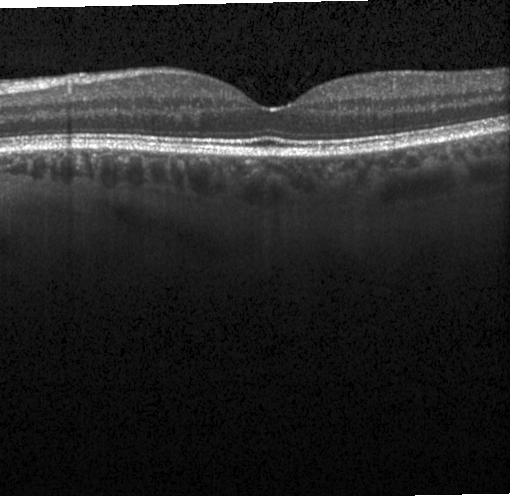
Fovea-centered, retinal OCT cross-section
Diagnosis: neither choroidal neovascularization, diabetic macular edema, nor drusen.